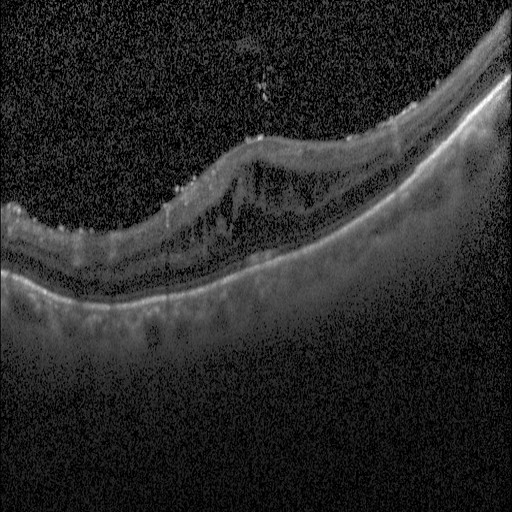 Finding: diabetic macular edema.